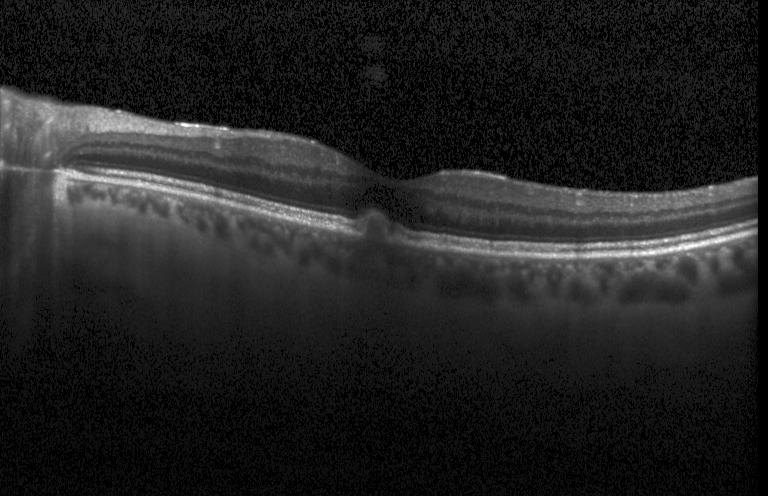
Diagnosis: sub-RPE drusenoid deposits.